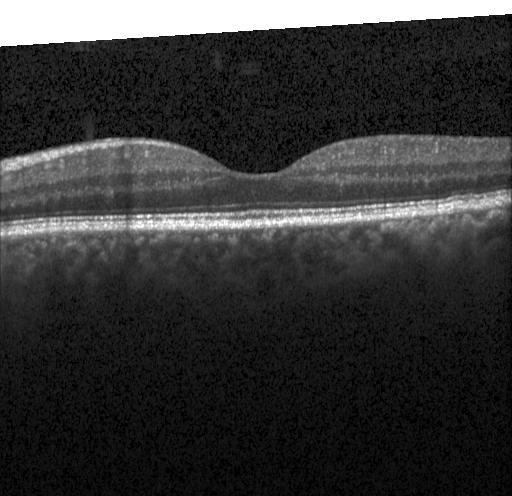

SD-OCT, OCT B-scan, acquired on a Heidelberg Spectralis, centered on the fovea — OCT finding: neither choroidal neovascularization, diabetic macular edema, nor drusen.